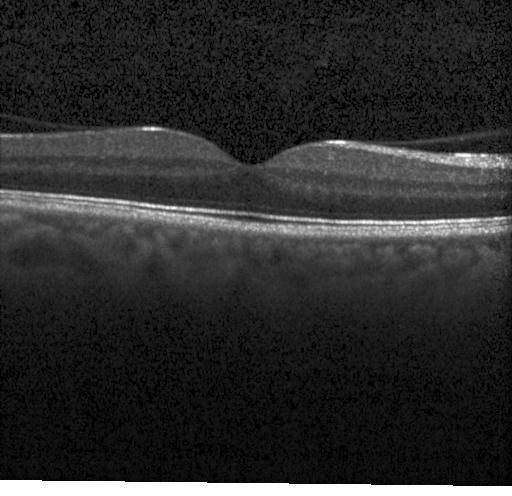
Dx: neither choroidal neovascularization, diabetic macular edema, nor drusen.